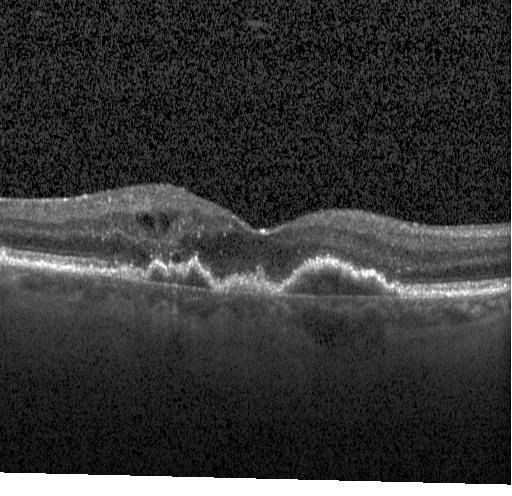
Dx: a choroidal neovascular membrane.